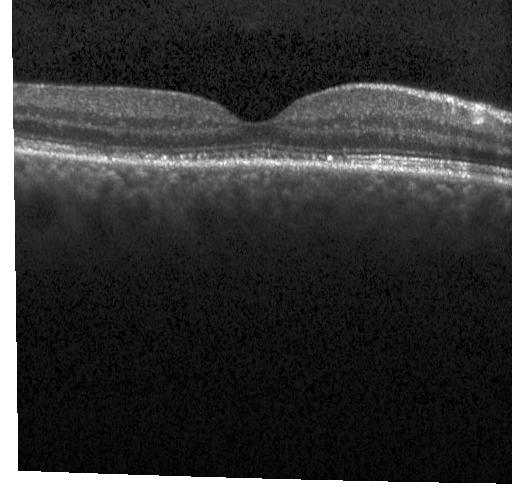

SD-OCT. Optical coherence tomography B-scan. Fovea-centered. Instrument: Heidelberg Spectralis
No evidence of choroidal neovascularization, diabetic macular edema, or drusen.